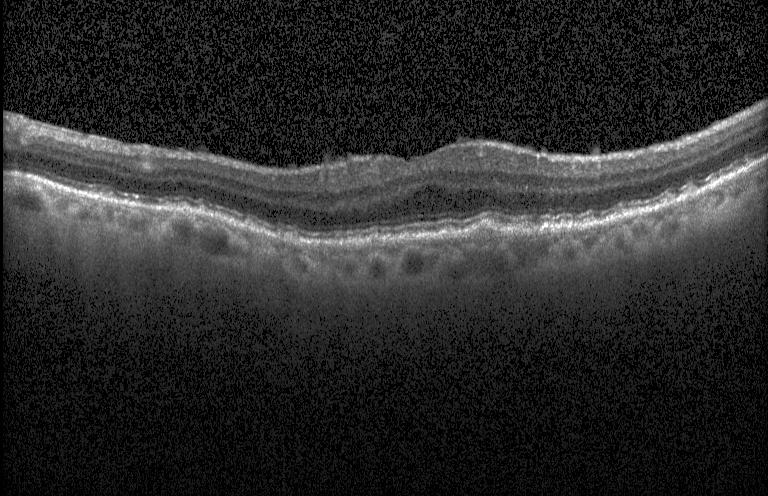
Spectral-domain optical coherence tomography; through the macula; retinal OCT cross-section; Heidelberg Spectralis. The scan shows drusen.